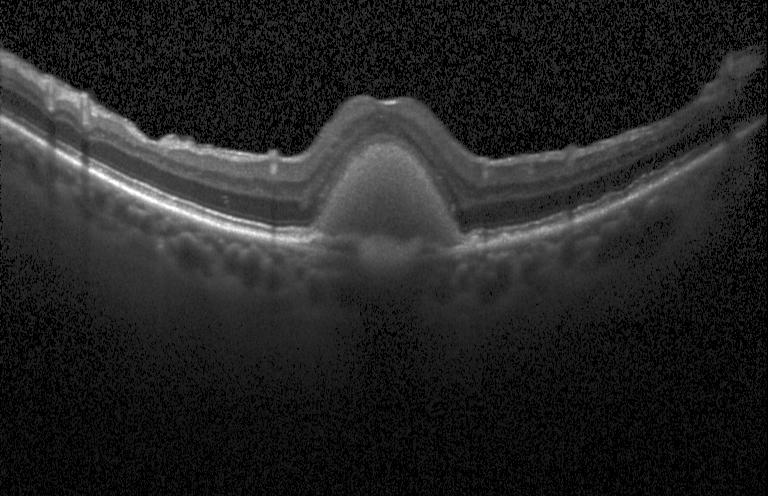 Spectral-domain optical coherence tomography · optical coherence tomography B-scan
Macular OCT: a choroidal neovascular membrane.